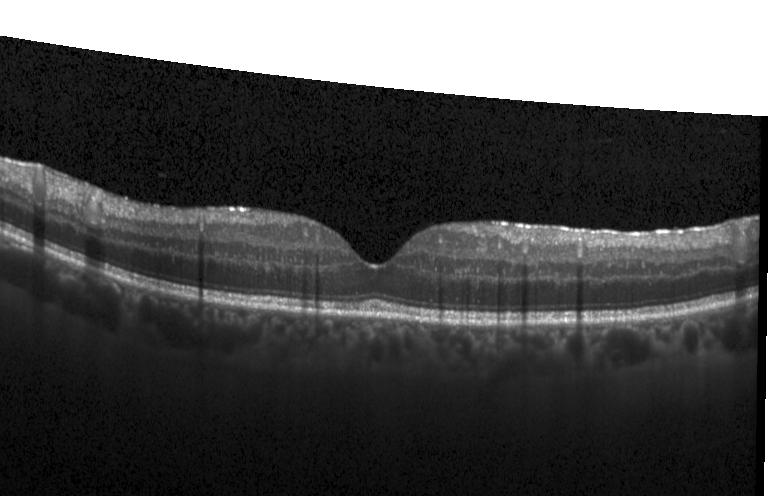

No evidence of choroidal neovascularization, diabetic macular edema, or drusen.